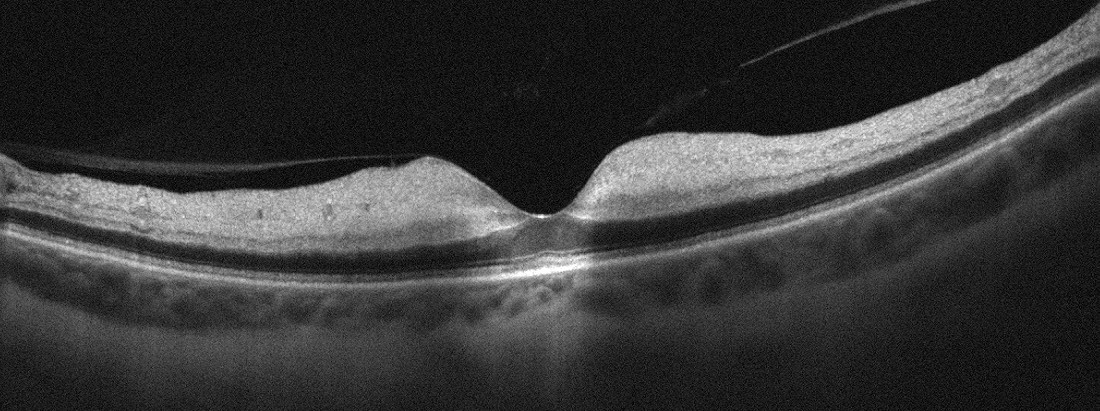
Retinal OCT cross-section
The scan shows RAO.